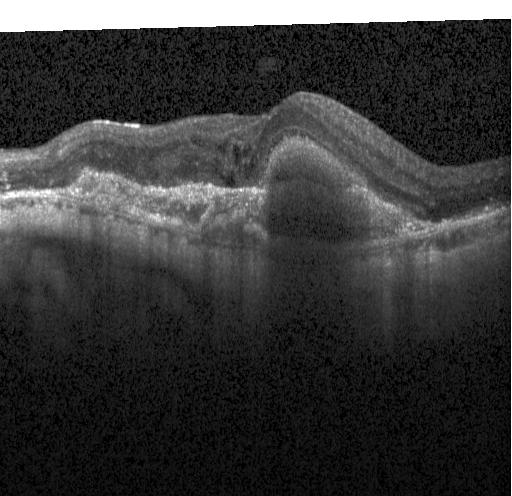 Impression: choroidal neovascularization (CNV).